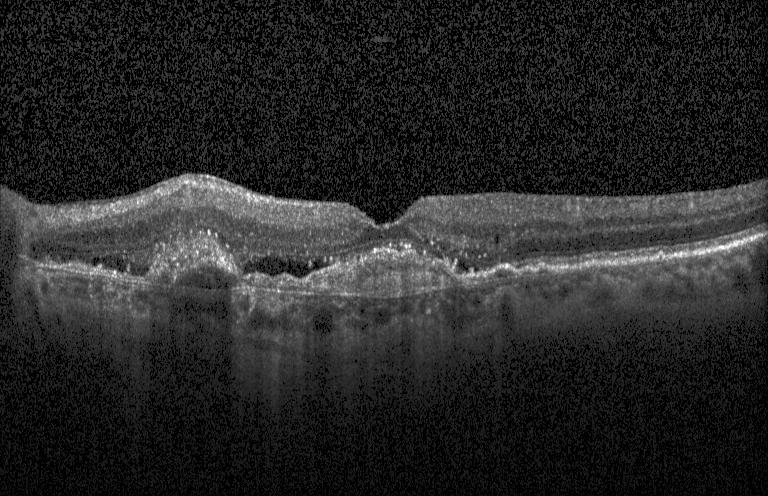

Impression: choroidal neovascularization.